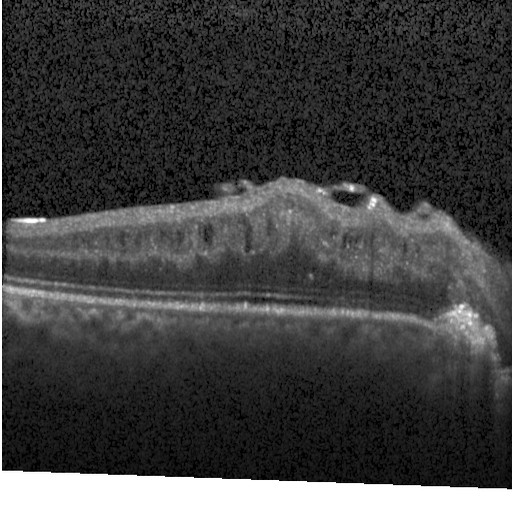
Diabetic macular edema (DME).